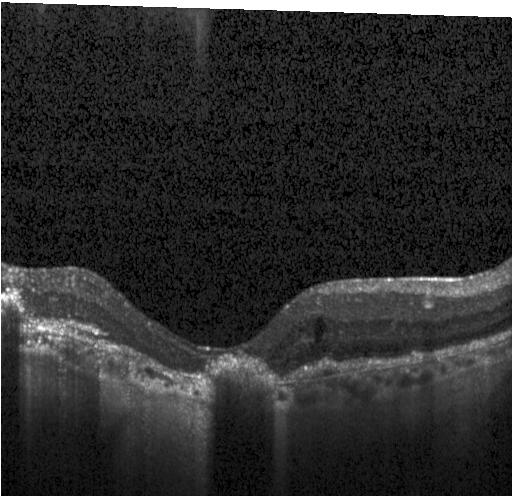
OCT B-scan — Finding: choroidal neovascularization.